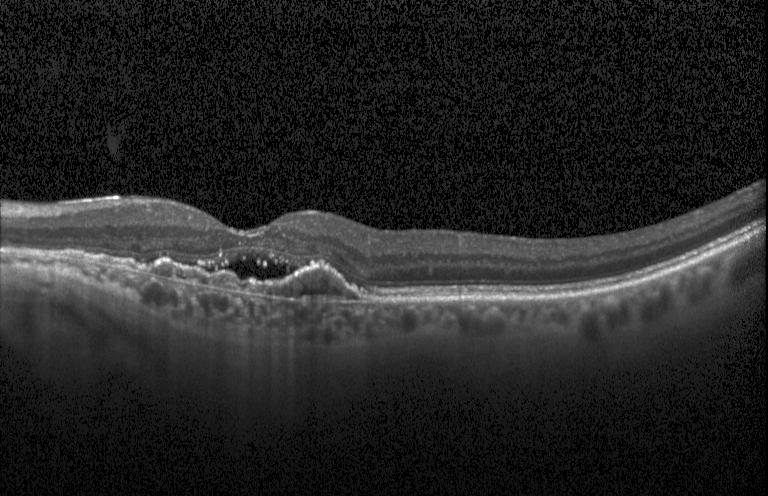
OCT line scan. Acquired on a Heidelberg Spectralis. Macular scan. SD-OCT
Finding: a choroidal neovascular membrane.